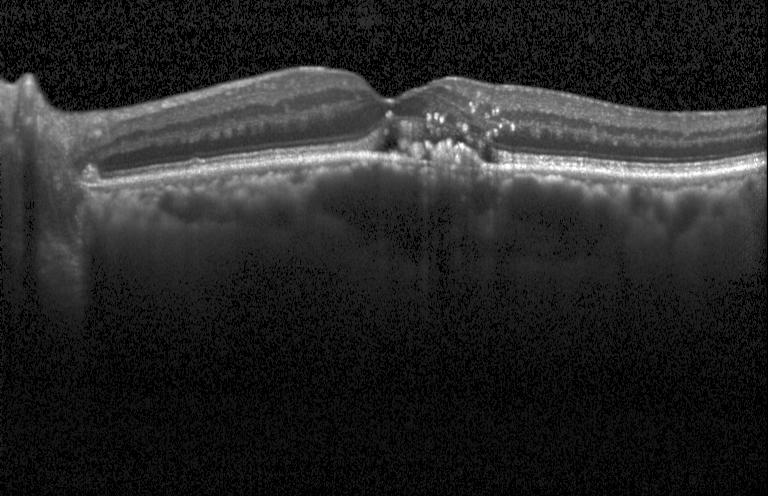 Retinal OCT cross-section, through the macula, spectral-domain optical coherence tomography.
Assessment: CNV.